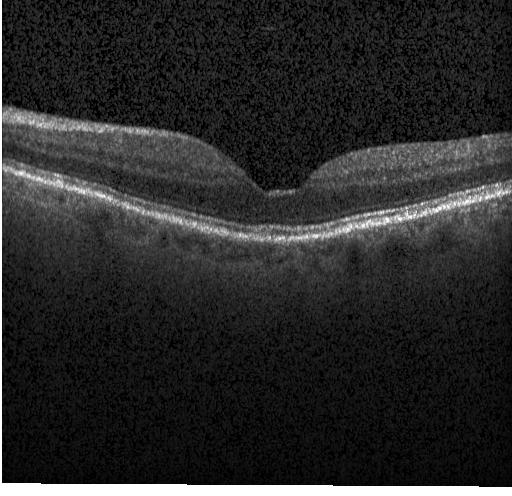

OCT B-scan · spectral-domain OCT.
Assessment: no CNV, no DME, and no drusen.